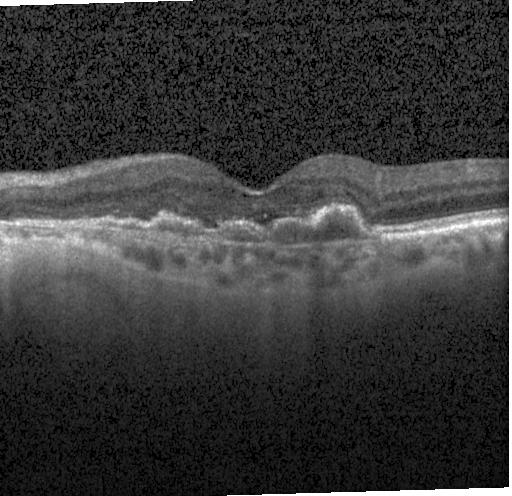

Spectral-domain OCT B-scan: CNV.